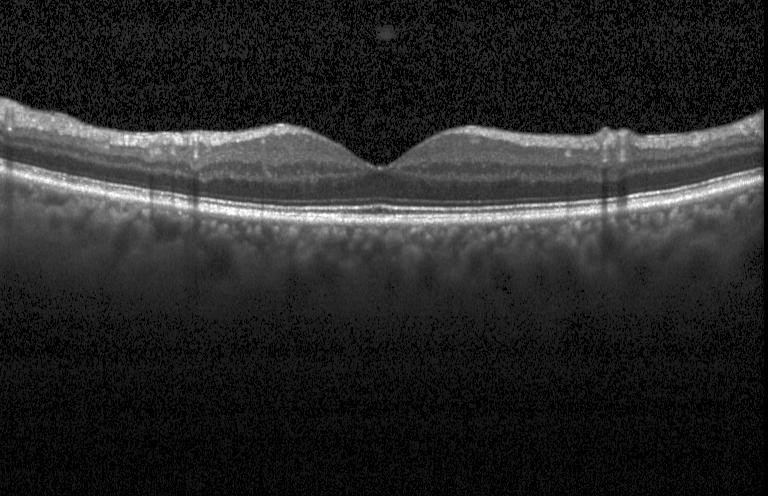

Spectral-domain OCT B-scan: neither choroidal neovascularization, diabetic macular edema, nor drusen.